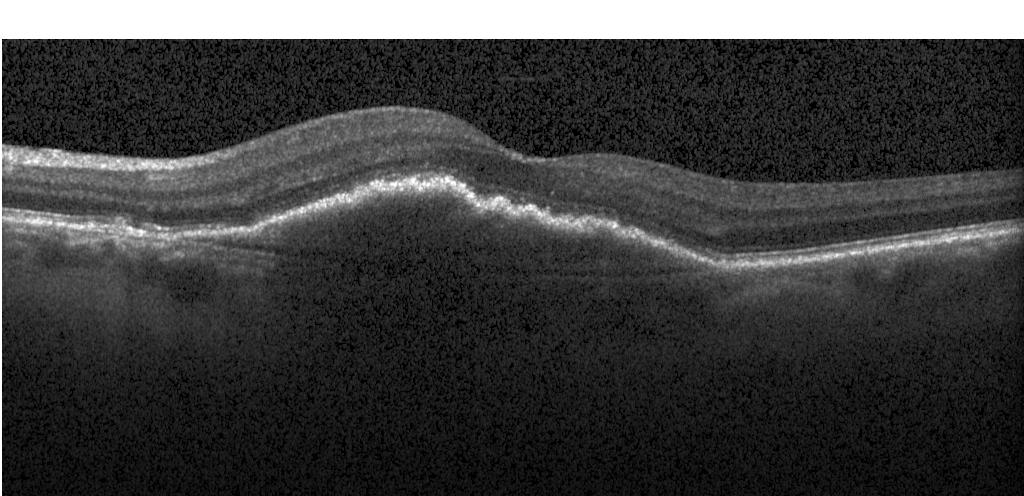
Macular OCT: a choroidal neovascular membrane.